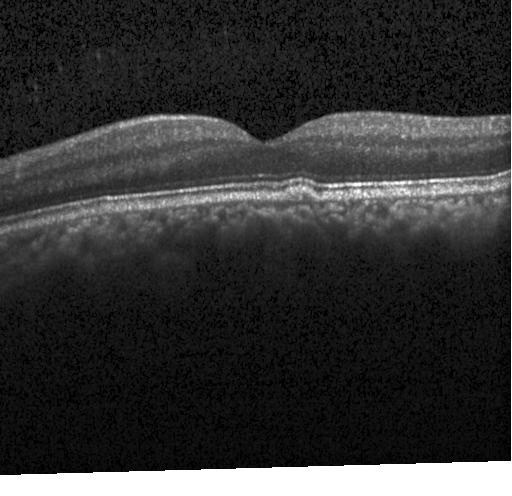

Spectral-domain optical coherence tomography, fovea-centered, Heidelberg Spectralis, retinal OCT B-scan — OCT finding: sub-RPE drusenoid deposits.